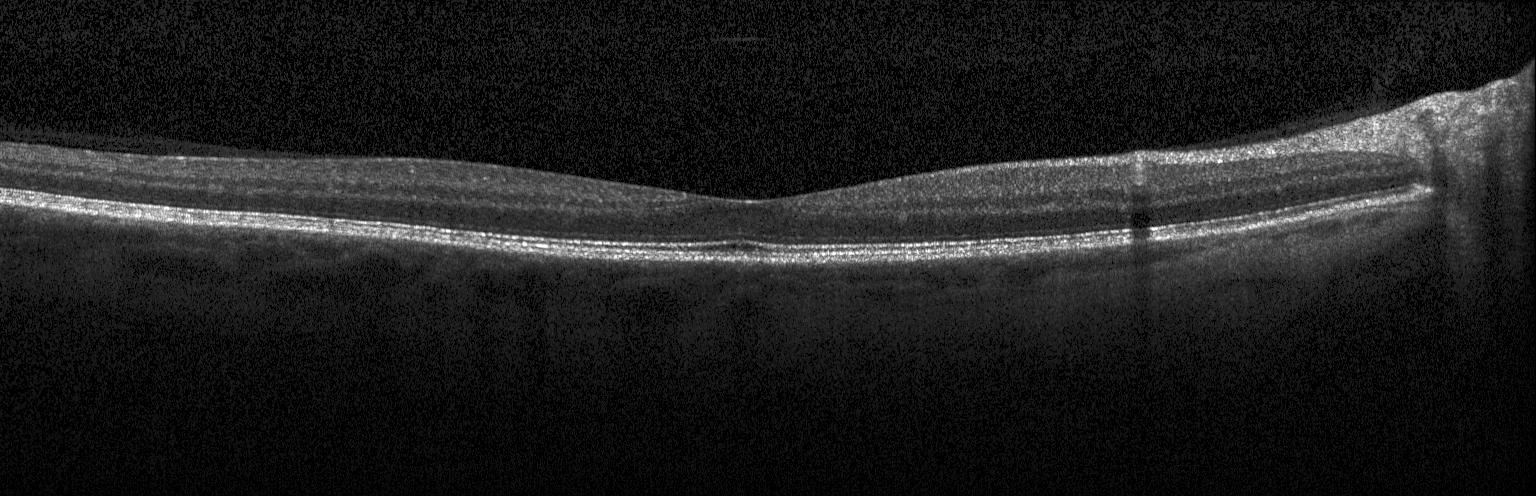

OCT B-scan showing no choroidal neovascularization, diabetic macular edema, or drusen.